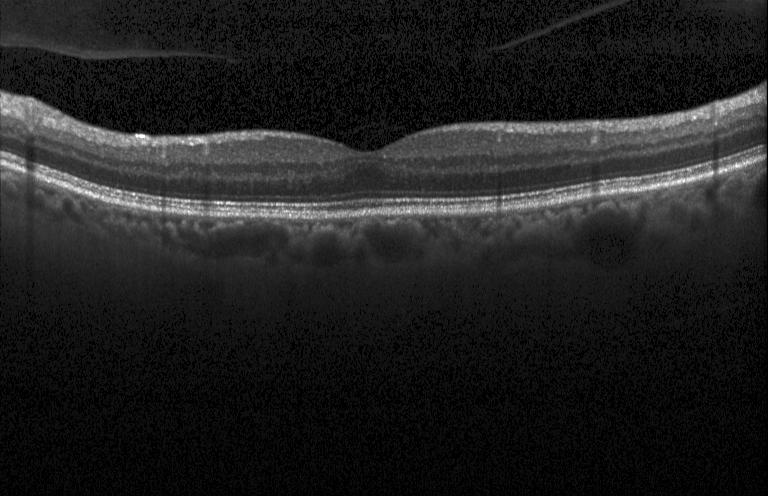
Optical coherence tomography B-scan. Heidelberg Spectralis OCT system.
Diagnosis: no choroidal neovascularization, no diabetic macular edema, and no drusen.